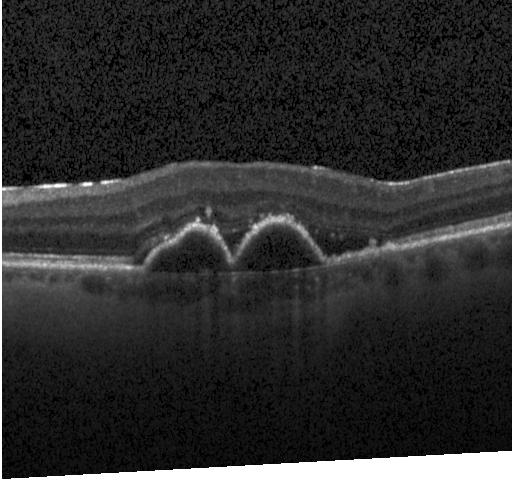

Optical coherence tomography B-scan — Impression: CNV.